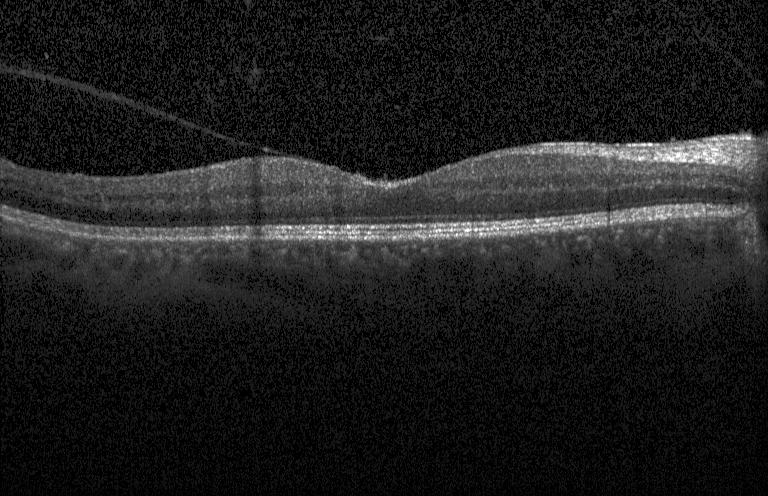

Macular OCT demonstrating no CNV, DME, or drusen.